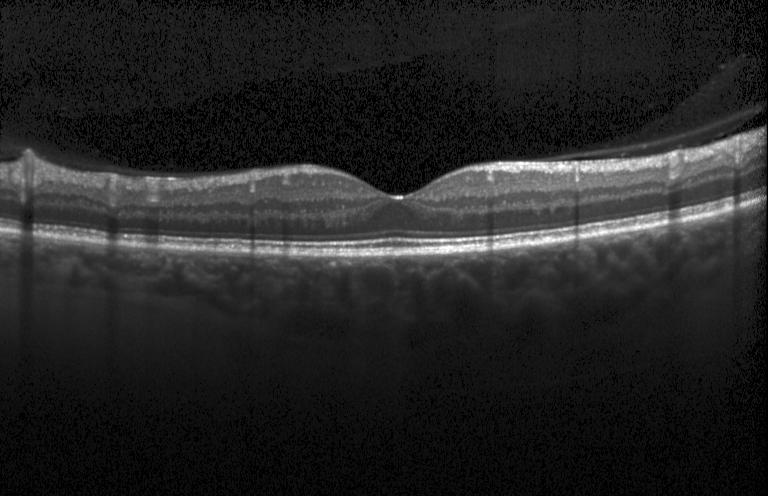
OCT B-scan · SD-OCT · horizontal scan through the fovea · instrument: Heidelberg Spectralis
Macular OCT: no CNV, DME, or drusen.